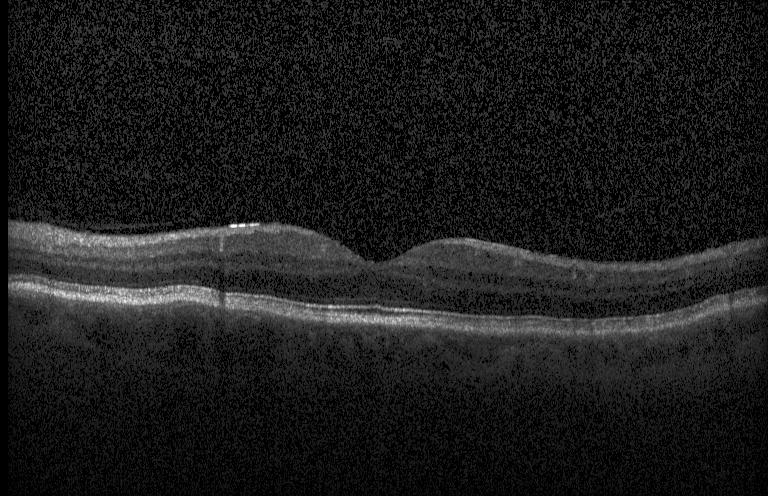

Retinal OCT cross-section. The scan shows neither choroidal neovascularization, diabetic macular edema, nor drusen.